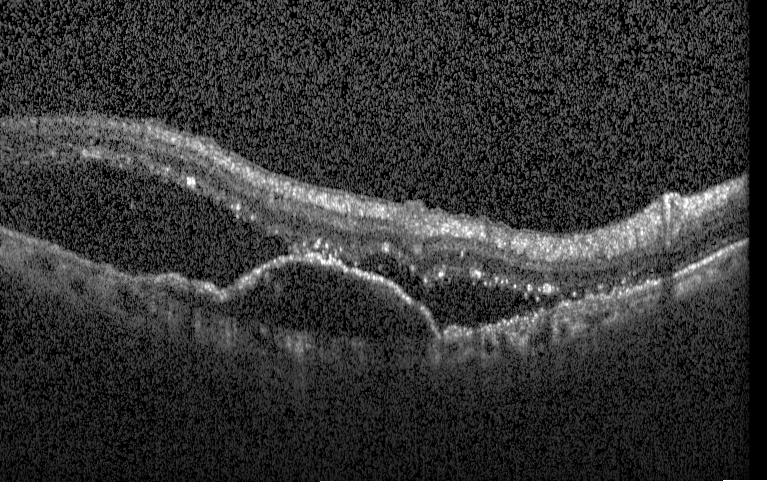

Diagnosis: a choroidal neovascular membrane.